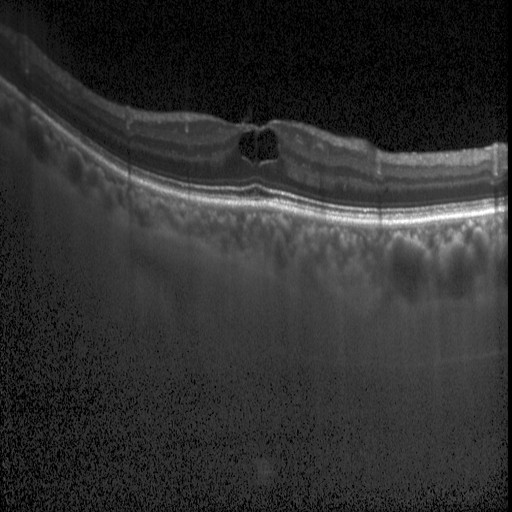

Retinal OCT cross-section · through the macula · Heidelberg Spectralis OCT system
Dx: diabetic macular edema (DME).